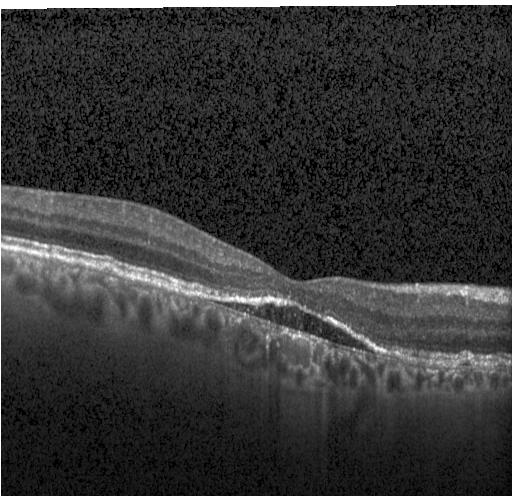

Macular scan; retinal OCT B-scan.
Impression: a choroidal neovascular membrane.